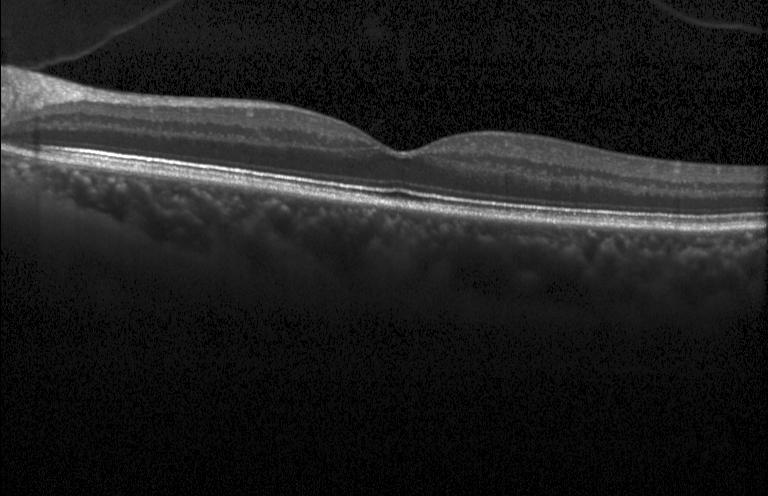

Spectral-domain OCT. Macular scan. Retinal OCT cross-section. Heidelberg Spectralis.
Neither CNV, DME, nor drusen.